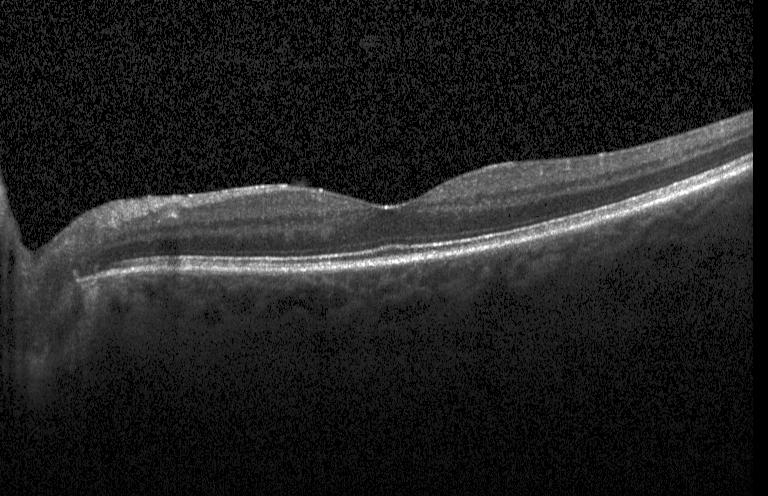
OCT line scan. Impression: no choroidal neovascularization, diabetic macular edema, or drusen.